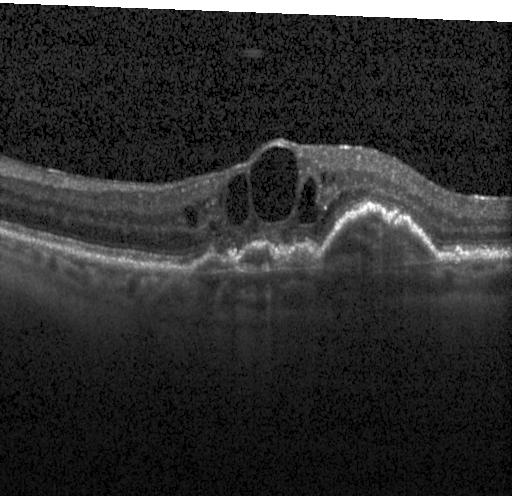
SD-OCT. Macular scan. Retinal OCT B-scan. Acquired on a Heidelberg Spectralis. This B-scan demonstrates a choroidal neovascular membrane.